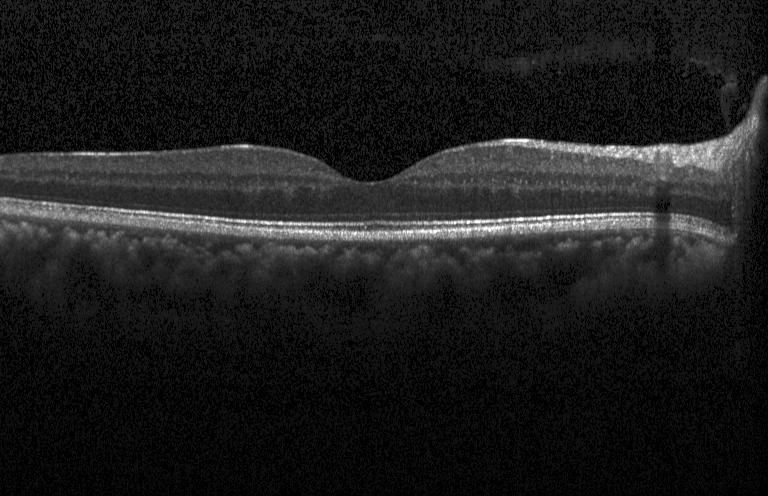
Diagnosis: no choroidal neovascularization, diabetic macular edema, or drusen.